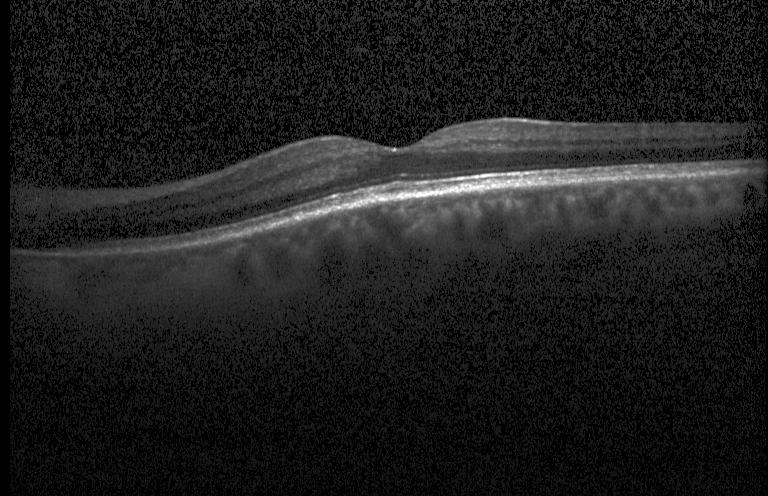

Spectral-domain OCT; horizontal scan through the fovea; optical coherence tomography B-scan; acquired on a Heidelberg Spectralis. No evidence of choroidal neovascularization, diabetic macular edema, or drusen.